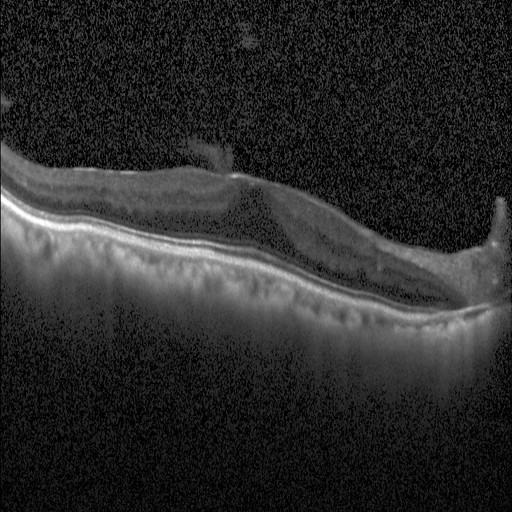
OCT B-scan; acquired on a Heidelberg Spectralis; fovea-centered; spectral-domain OCT.
Dx: diabetic macular edema.